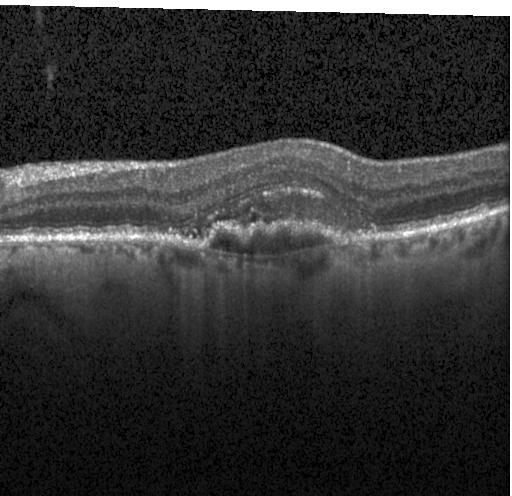

OCT B-scan showing a choroidal neovascular membrane.